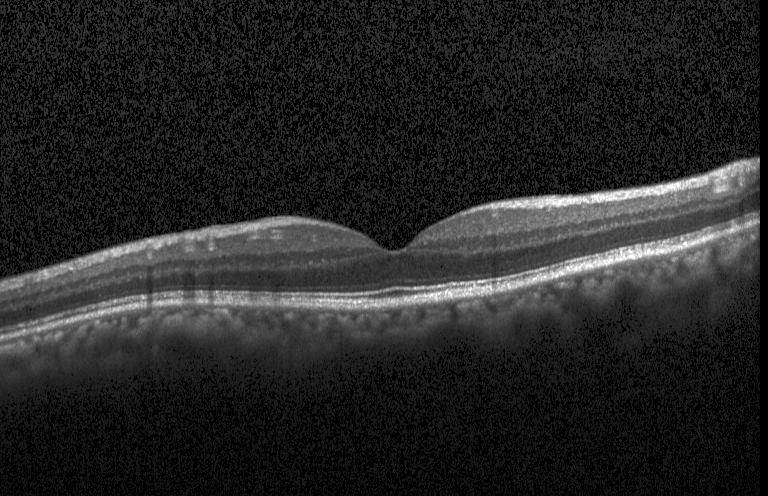 Spectral-domain OCT; through the macula; optical coherence tomography B-scan; Heidelberg Spectralis
OCT finding: no choroidal neovascularization, no diabetic macular edema, and no drusen.